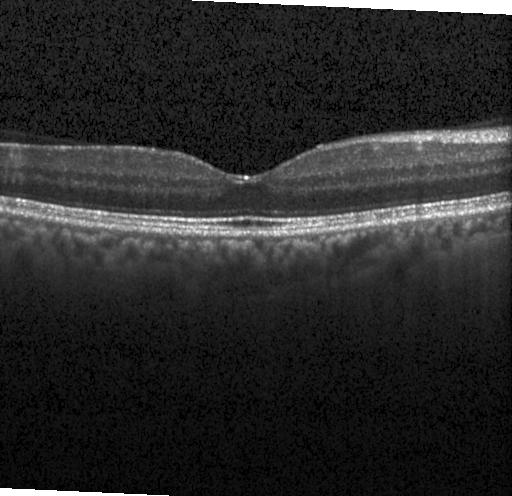 SD-OCT · OCT B-scan · Heidelberg Spectralis.
Dx: no CNV, DME, or drusen.